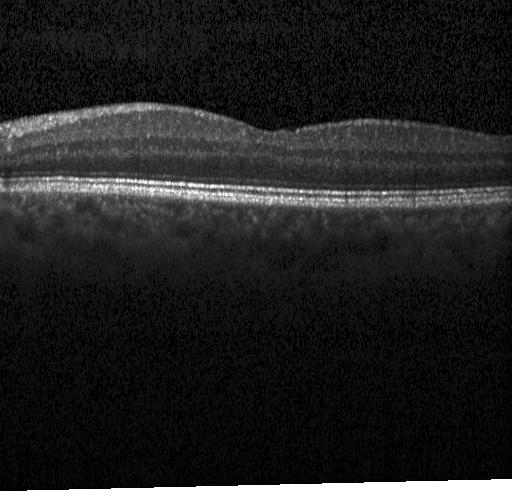 Optical coherence tomography B-scan. OCT finding: no choroidal neovascularization, no diabetic macular edema, and no drusen.